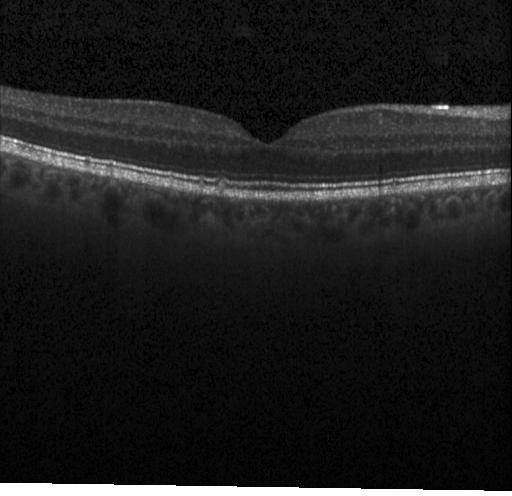

Retinal OCT B-scan · spectral-domain OCT · macular scan — Assessment: sub-RPE drusenoid deposits.